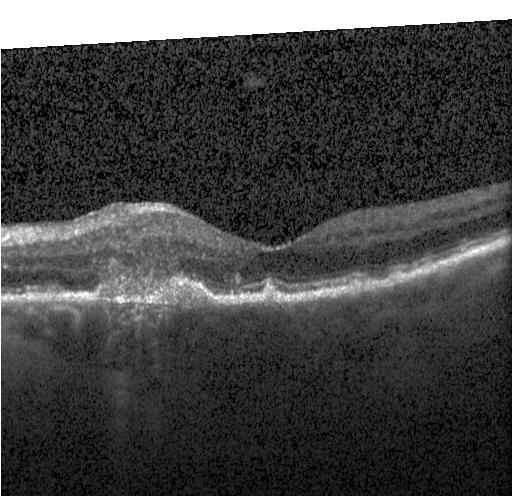 Impression: CNV.